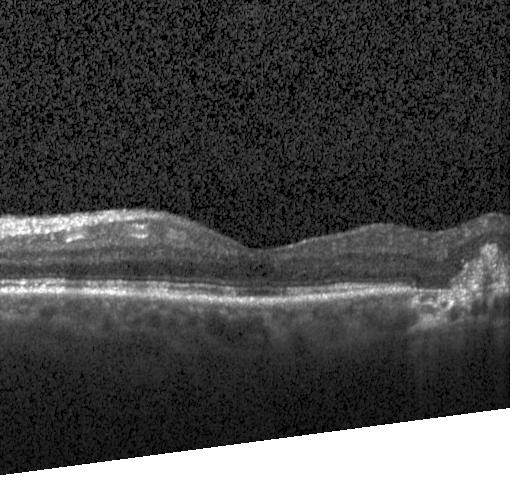

OCT B-scan showing CNV.